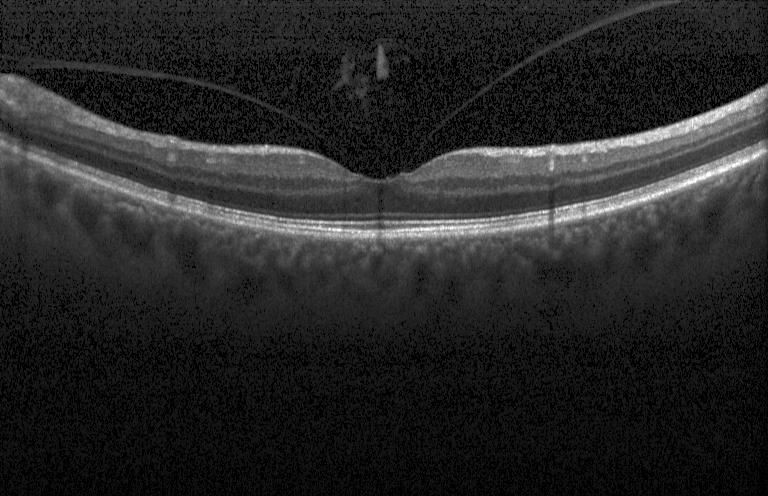
Retinal OCT cross-section showing no choroidal neovascularization, diabetic macular edema, or drusen.